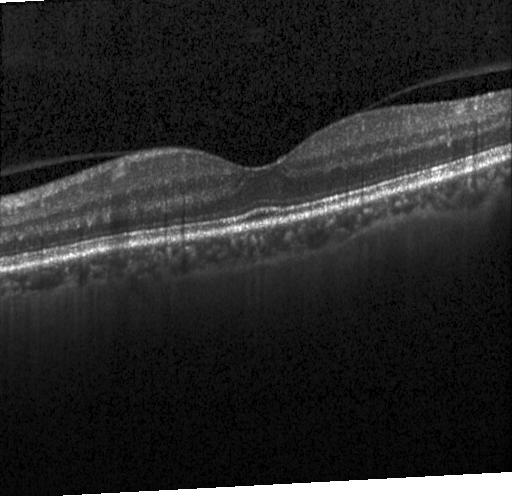 Fovea-centered; Heidelberg Spectralis OCT system; spectral-domain optical coherence tomography; optical coherence tomography scan.
Macular OCT: no CNV, DME, or drusen.